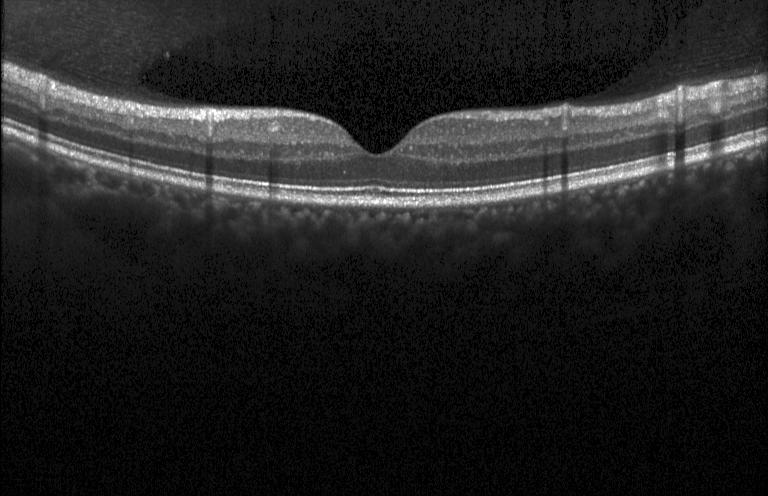
Instrument: Heidelberg Spectralis · retinal OCT cross-section · through the macula · spectral-domain OCT — Diagnosis: no CNV, no DME, and no drusen.